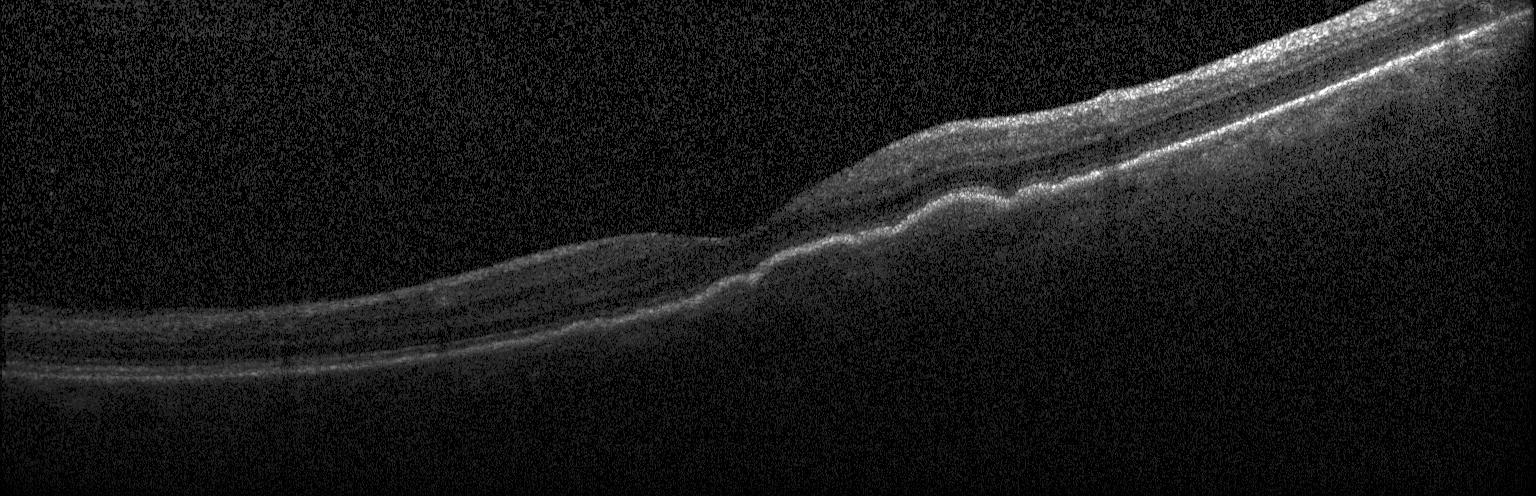
Spectral-domain optical coherence tomography, Heidelberg Spectralis OCT system, retinal OCT B-scan, macular scan.
The scan shows a choroidal neovascular membrane.